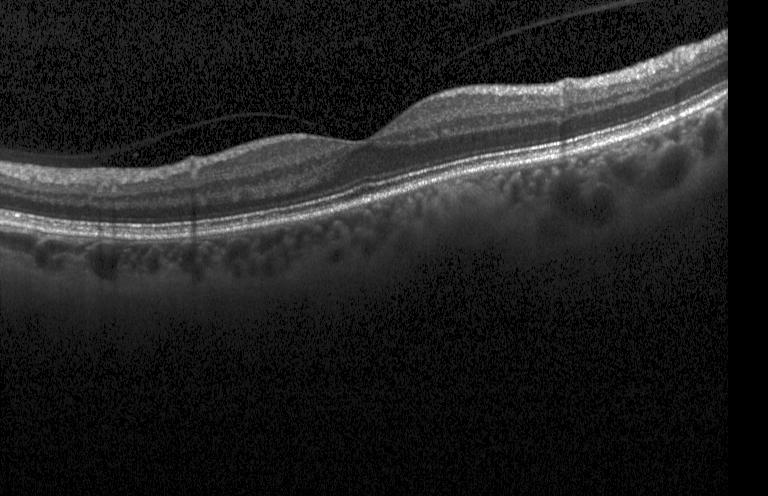

Instrument: Heidelberg Spectralis, OCT B-scan.
Diagnosis: no choroidal neovascularization, no diabetic macular edema, and no drusen.